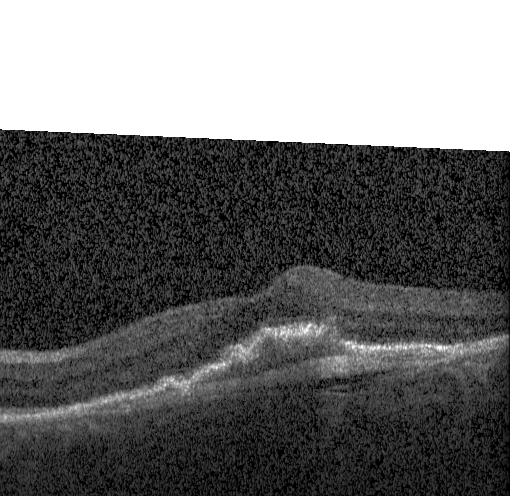

OCT line scan
The scan shows CNV.